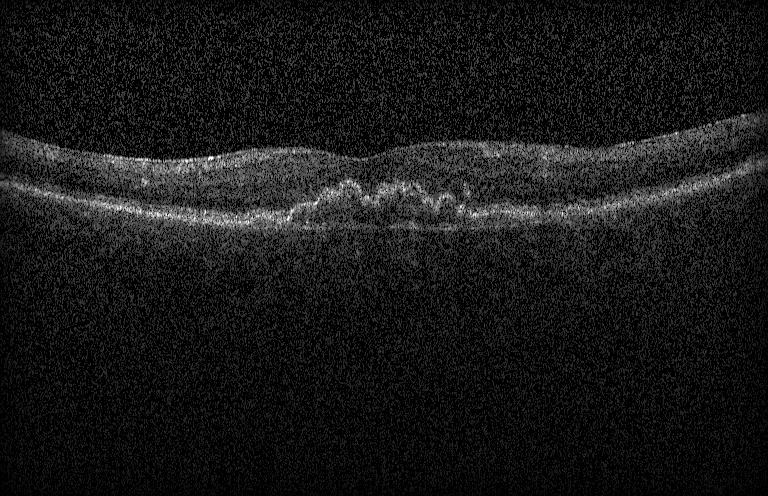 Retinal OCT cross-section · fovea-centered.
Macular OCT: CNV.